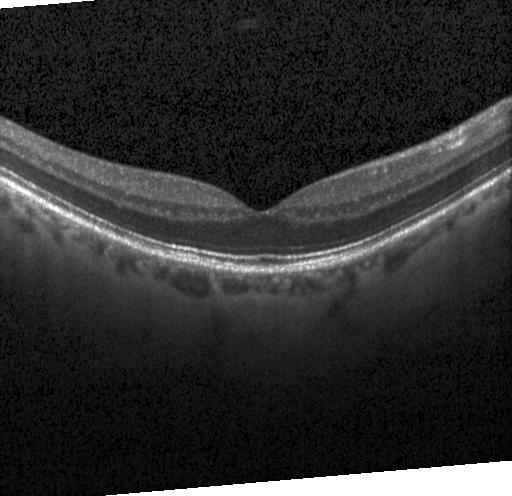 No CNV, DME, or drusen.